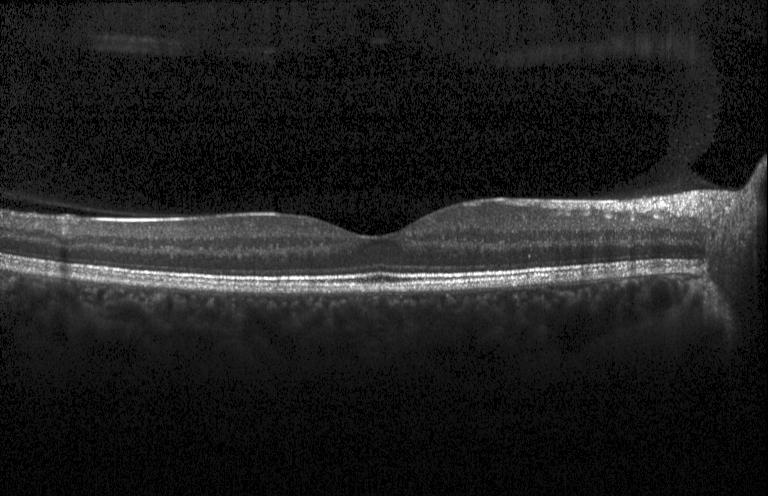

Through the macula · acquired on a Heidelberg Spectralis · OCT B-scan · SD-OCT
Impression: neither choroidal neovascularization, diabetic macular edema, nor drusen.